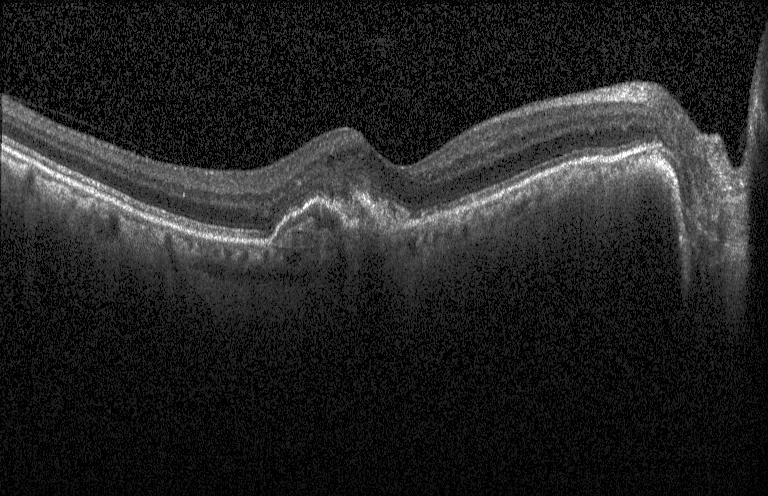 Optical coherence tomography scan; Heidelberg Spectralis OCT system; spectral-domain OCT; horizontal scan through the fovea. Impression: a choroidal neovascular membrane.